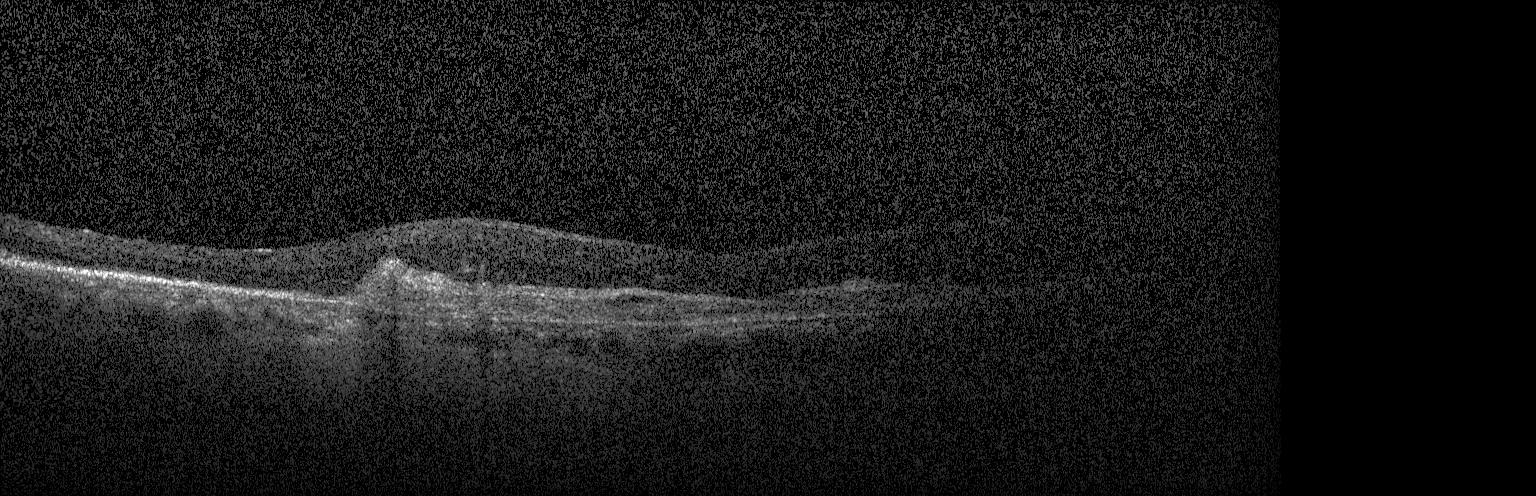

OCT line scan; SD-OCT. Finding: a choroidal neovascular membrane.